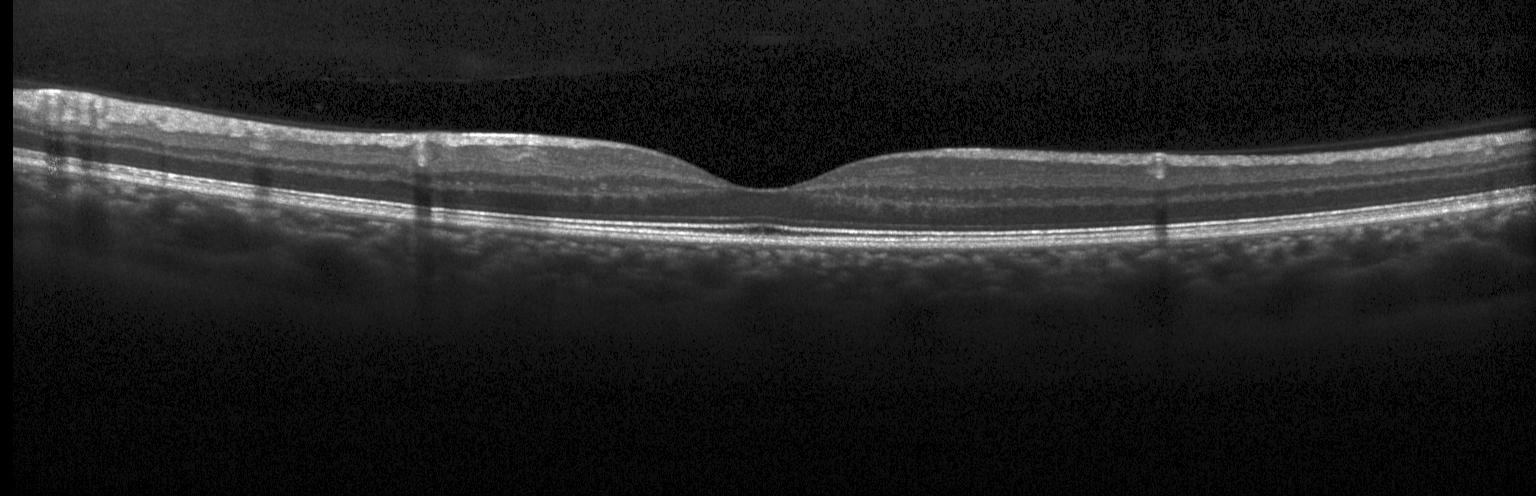

OCT B-scan · horizontal scan through the fovea · SD-OCT · Heidelberg Spectralis.
No evidence of CNV, DME, or drusen.